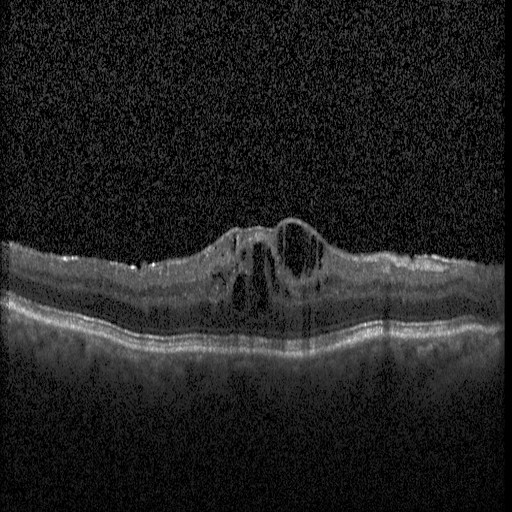
Optical coherence tomography B-scan — The scan shows diabetic macular edema (DME).